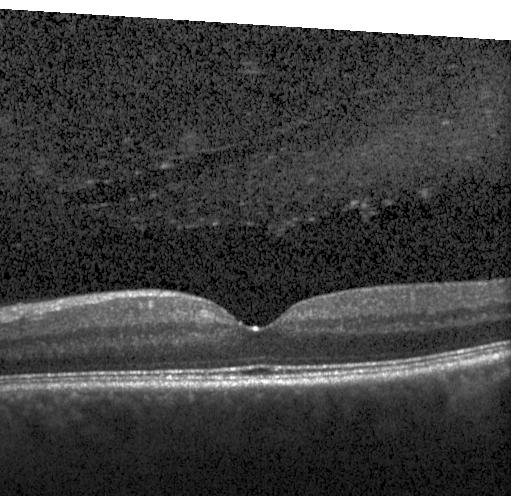

Through the macula. Optical coherence tomography scan. Spectral-domain OCT. Heidelberg Spectralis — The scan shows neither choroidal neovascularization, diabetic macular edema, nor drusen.